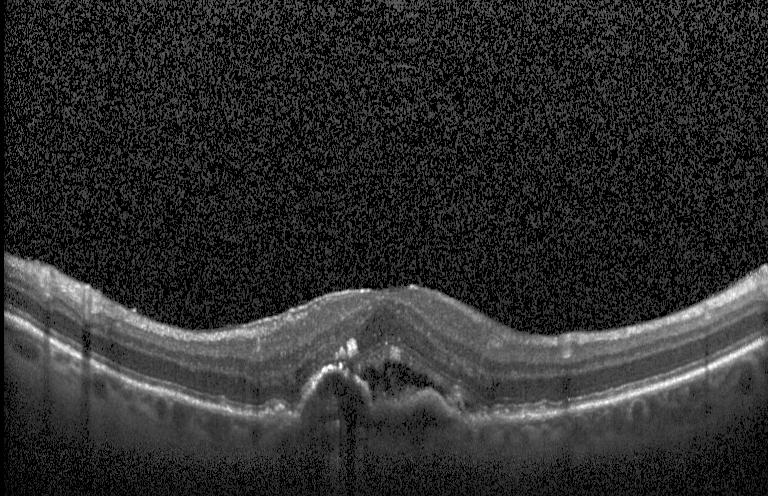
OCT B-scan. Impression: a choroidal neovascular membrane.